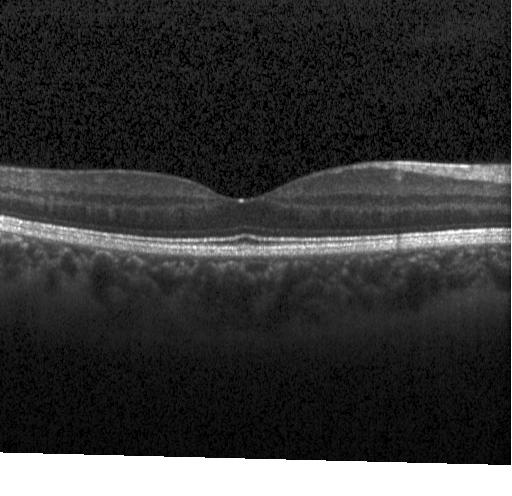
Retinal OCT cross-section showing no choroidal neovascularization, diabetic macular edema, or drusen.